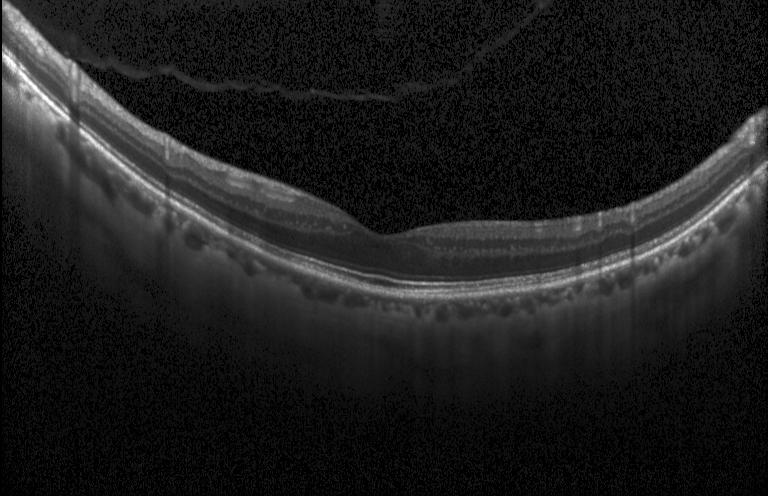
Through the macula; retinal OCT B-scan; spectral-domain OCT — This B-scan demonstrates no evidence of CNV, DME, or drusen.